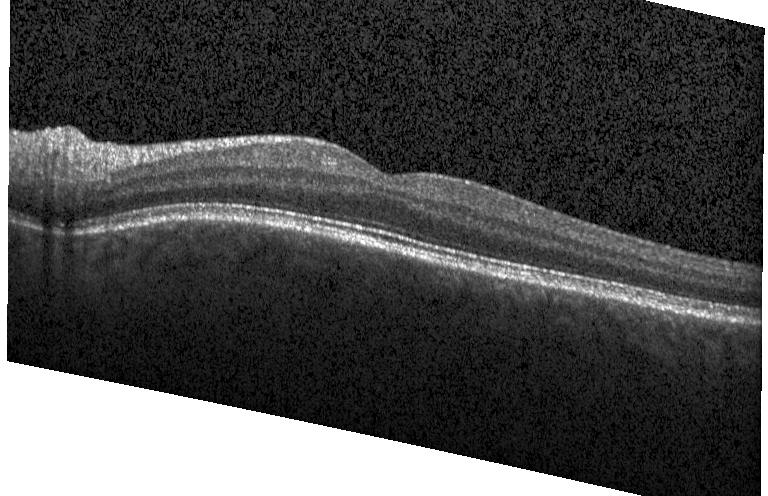 This B-scan demonstrates no CNV, DME, or drusen.